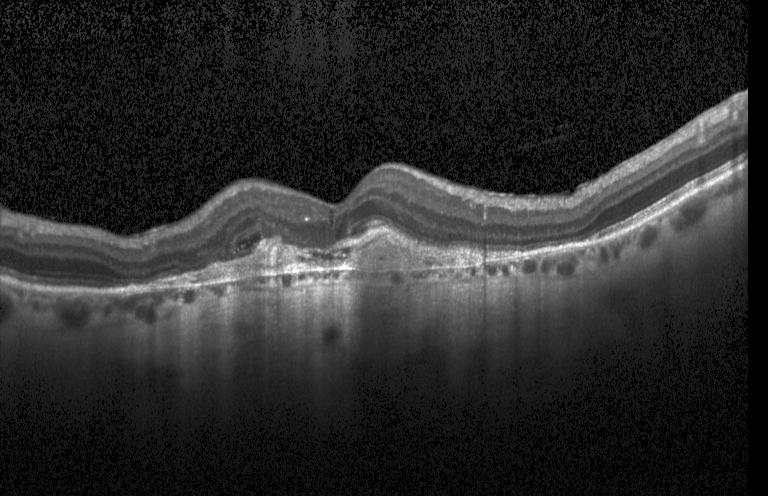 Finding: a choroidal neovascular membrane.